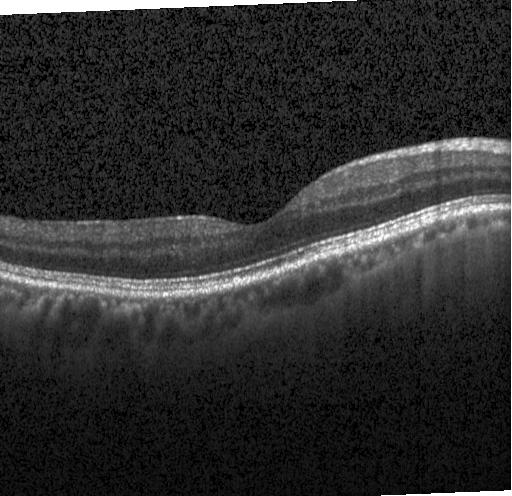

Optical coherence tomography B-scan; SD-OCT. Assessment: no choroidal neovascularization, no diabetic macular edema, and no drusen.